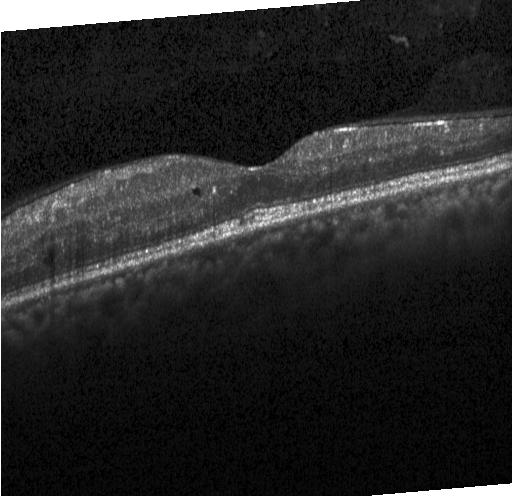
OCT line scan. DME.